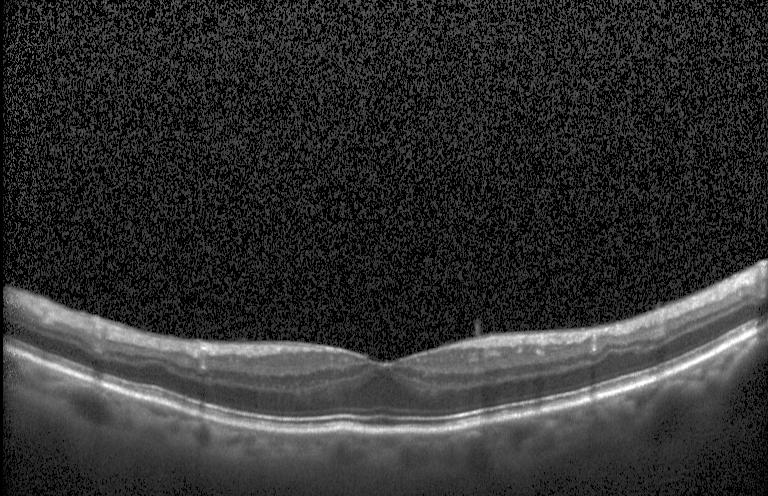
Macular OCT demonstrating neither choroidal neovascularization, diabetic macular edema, nor drusen.